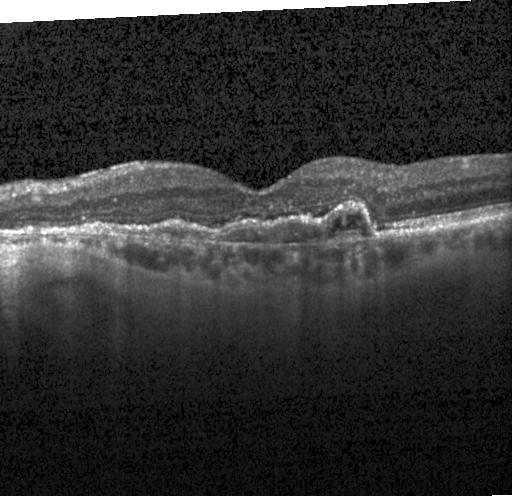

Diagnosis: choroidal neovascularization.